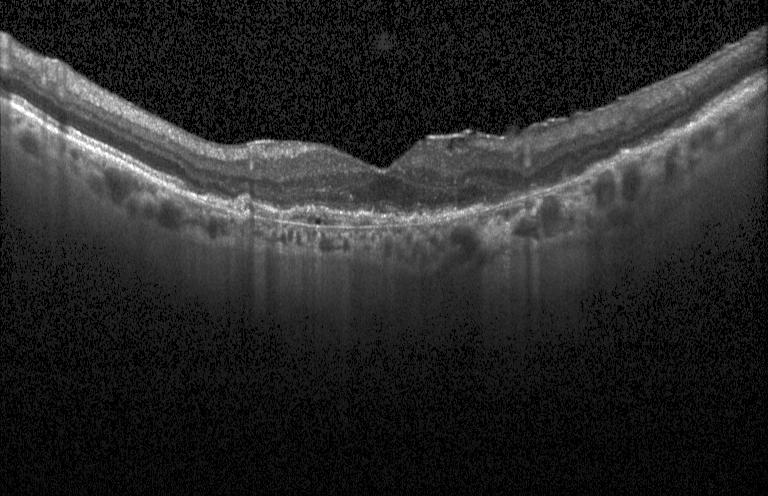
The scan shows choroidal neovascularization.